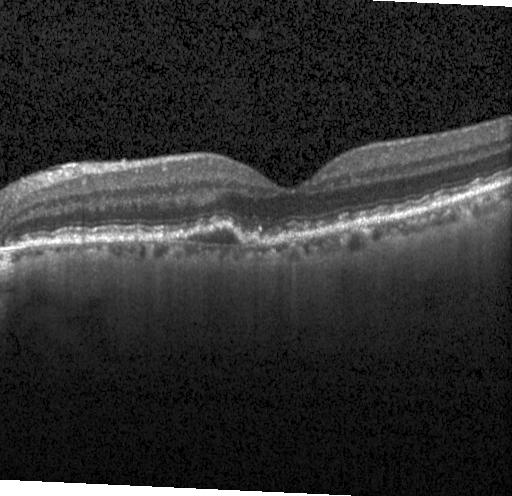

Through the macula. Optical coherence tomography scan
Diagnosis: CNV.